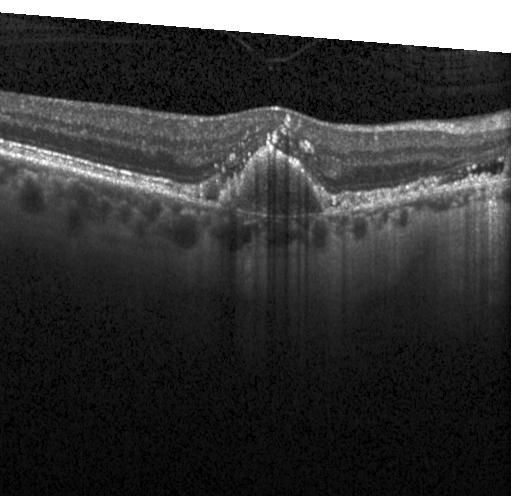

This B-scan demonstrates choroidal neovascularization.